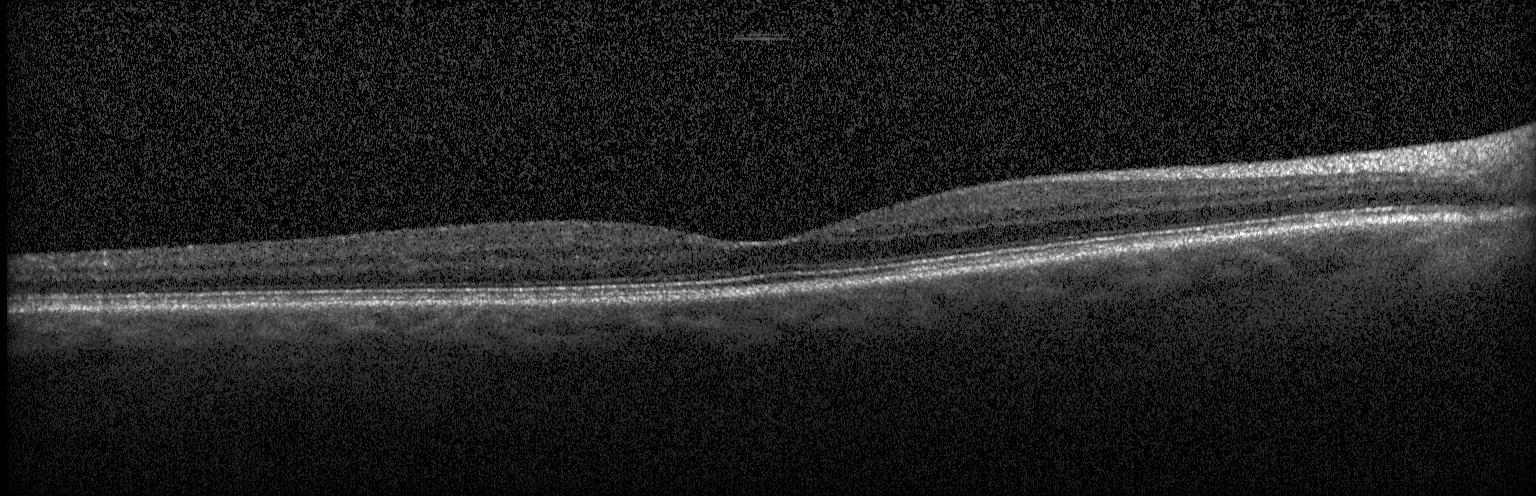 Instrument: Heidelberg Spectralis · OCT line scan · macular scan · spectral-domain optical coherence tomography.
Impression: no choroidal neovascularization, no diabetic macular edema, and no drusen.